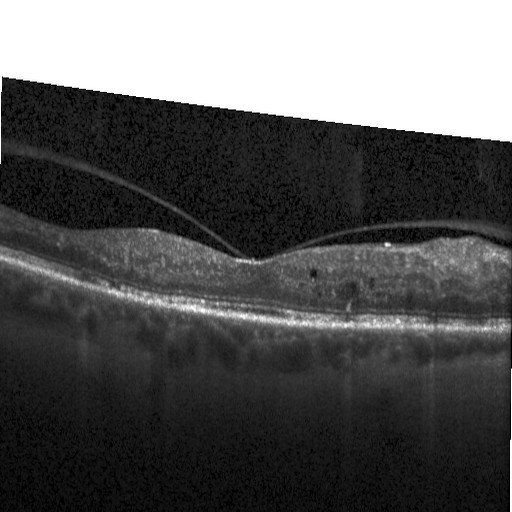

Finding: DME.